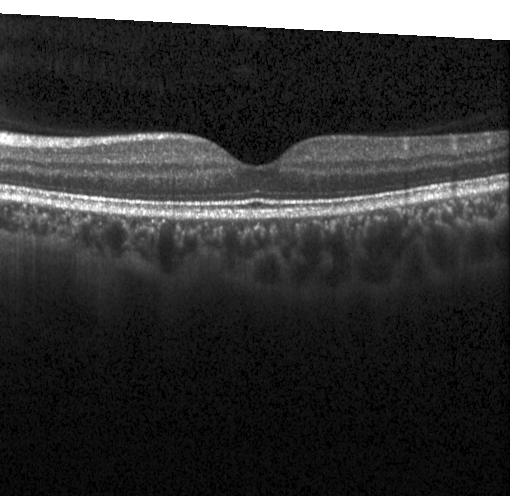
SD-OCT, retinal OCT B-scan, acquired on a Heidelberg Spectralis — Finding: no choroidal neovascularization, no diabetic macular edema, and no drusen.